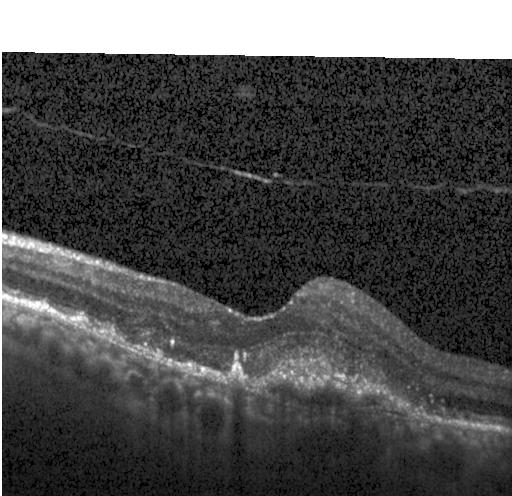

Macular OCT demonstrating a choroidal neovascular membrane.